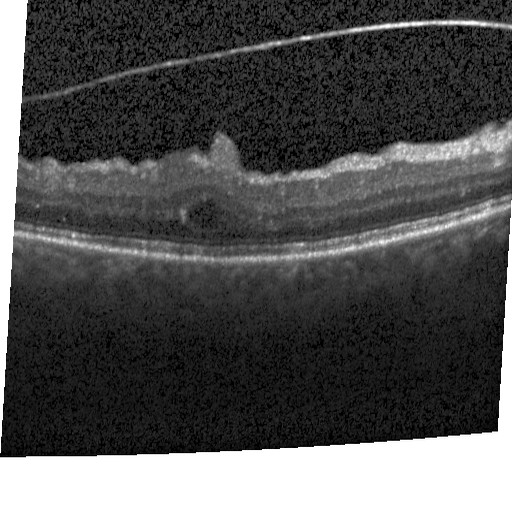

Optical coherence tomography scan · Heidelberg Spectralis OCT system — Diagnosis: diabetic macular edema.